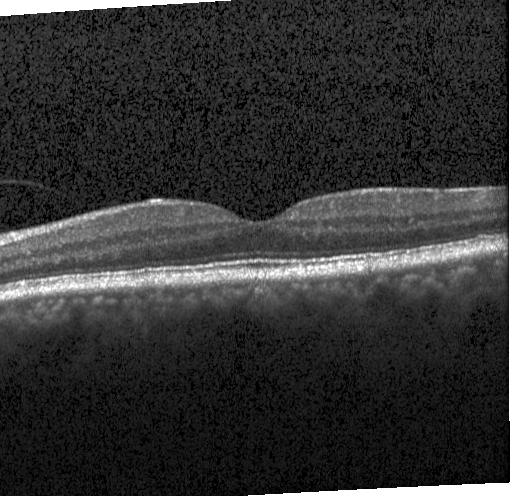
Spectral-domain OCT, OCT B-scan, through the macula, instrument: Heidelberg Spectralis.
The scan shows neither CNV, DME, nor drusen.